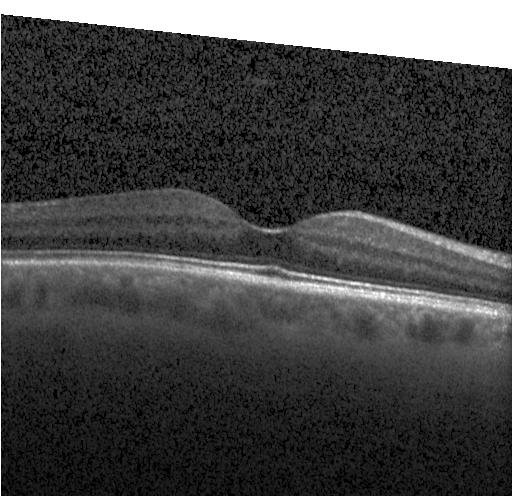 Macular OCT demonstrating no CNV, no DME, and no drusen.